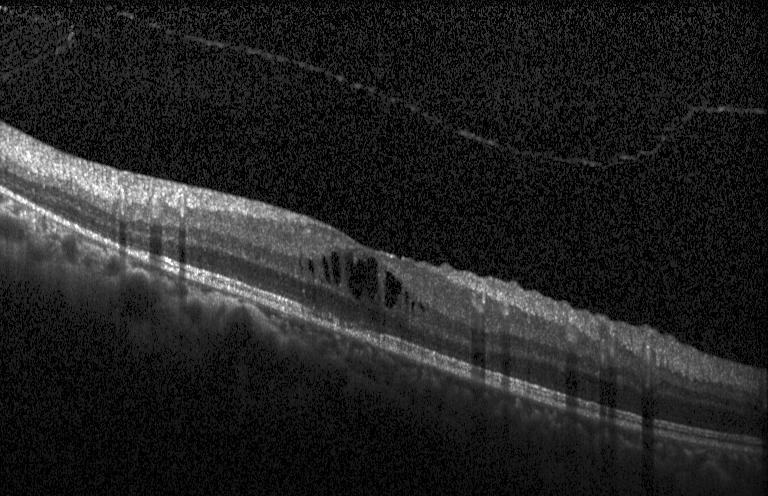 OCT line scan; fovea-centered; acquired on a Heidelberg Spectralis. The scan shows diabetic macular edema.